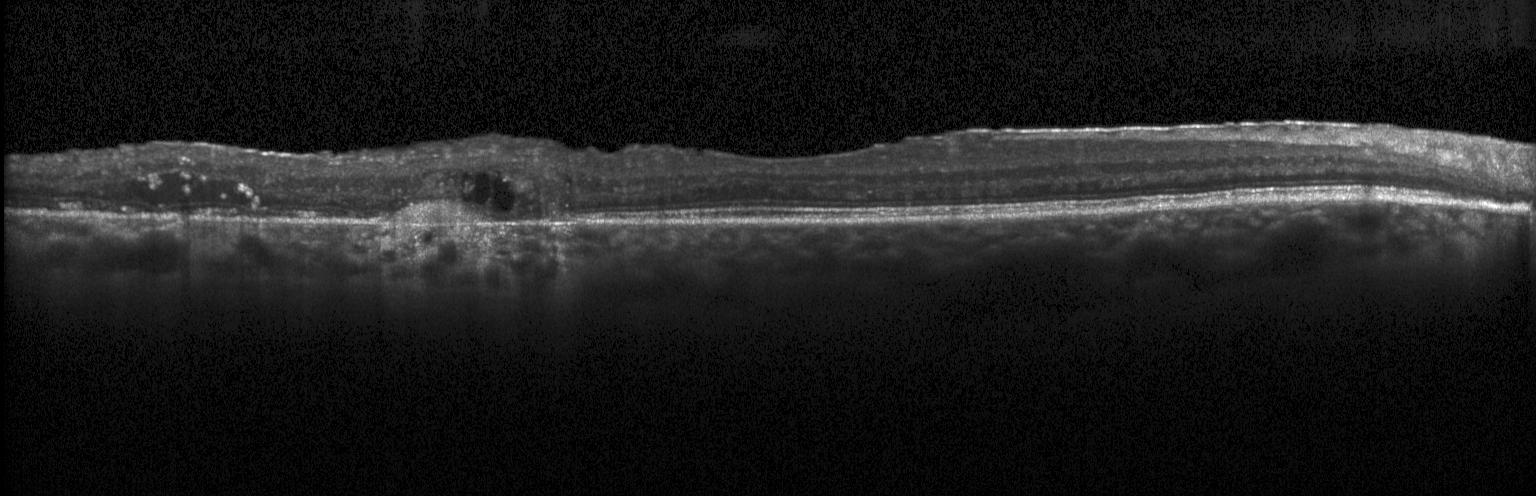 Spectral-domain OCT B-scan: a choroidal neovascular membrane.